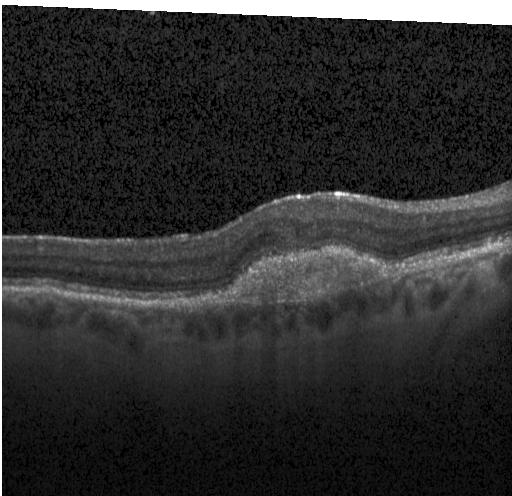
The scan shows a choroidal neovascular membrane.